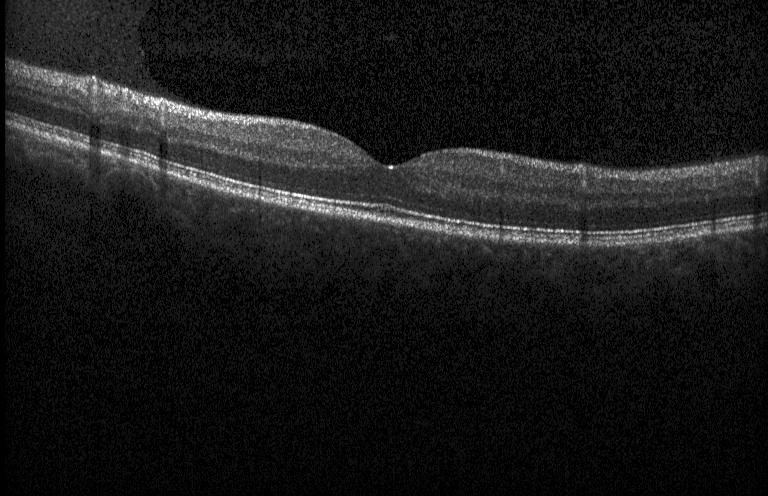

OCT line scan.
No evidence of choroidal neovascularization, diabetic macular edema, or drusen.